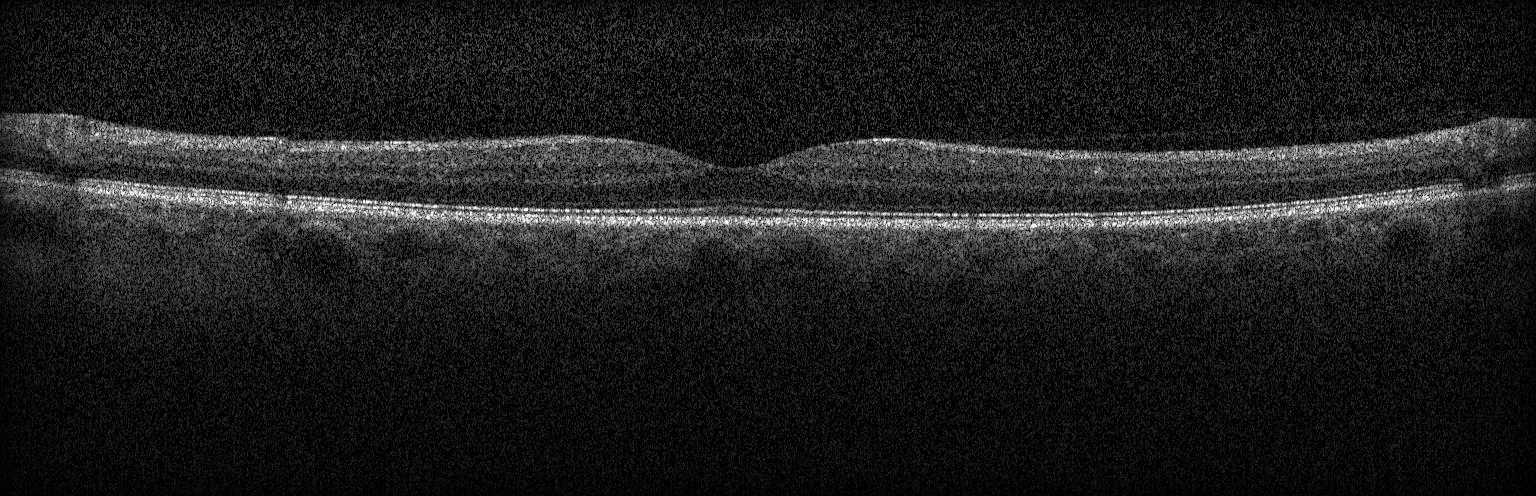
Acquired on a Heidelberg Spectralis, optical coherence tomography scan, through the macula, SD-OCT
Dx: no choroidal neovascularization, no diabetic macular edema, and no drusen.